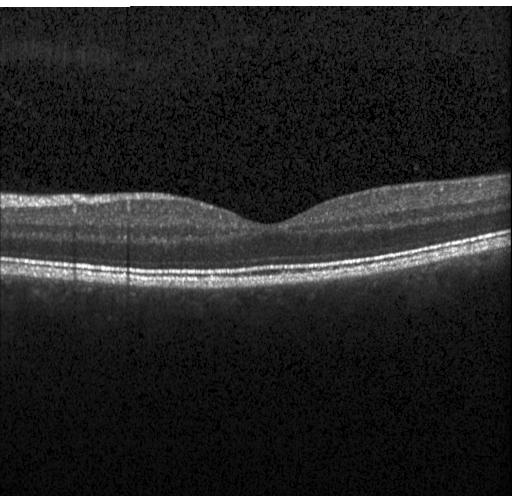
Optical coherence tomography B-scan. Horizontal scan through the fovea. Acquired on a Heidelberg Spectralis. SD-OCT. OCT finding: neither choroidal neovascularization, diabetic macular edema, nor drusen.